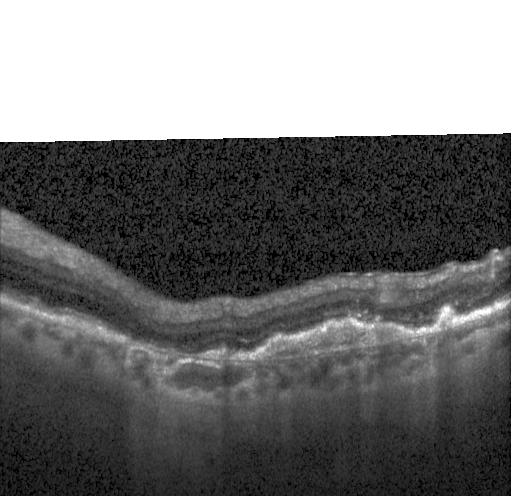 Spectral-domain optical coherence tomography · macular scan · acquired on a Heidelberg Spectralis · optical coherence tomography scan — Choroidal neovascularization (CNV).